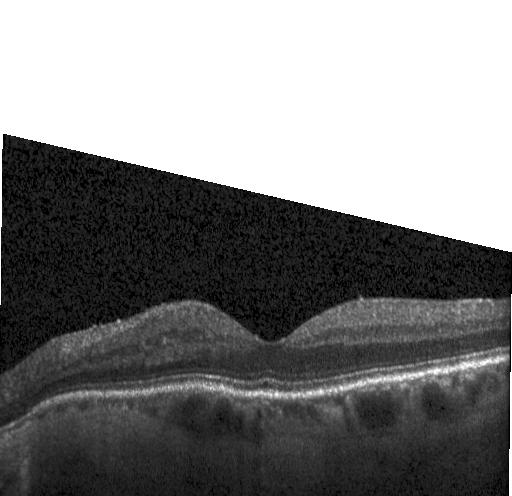
Heidelberg Spectralis. Spectral-domain optical coherence tomography. Retinal OCT B-scan. Through the macula.
This B-scan demonstrates no choroidal neovascularization, no diabetic macular edema, and no drusen.